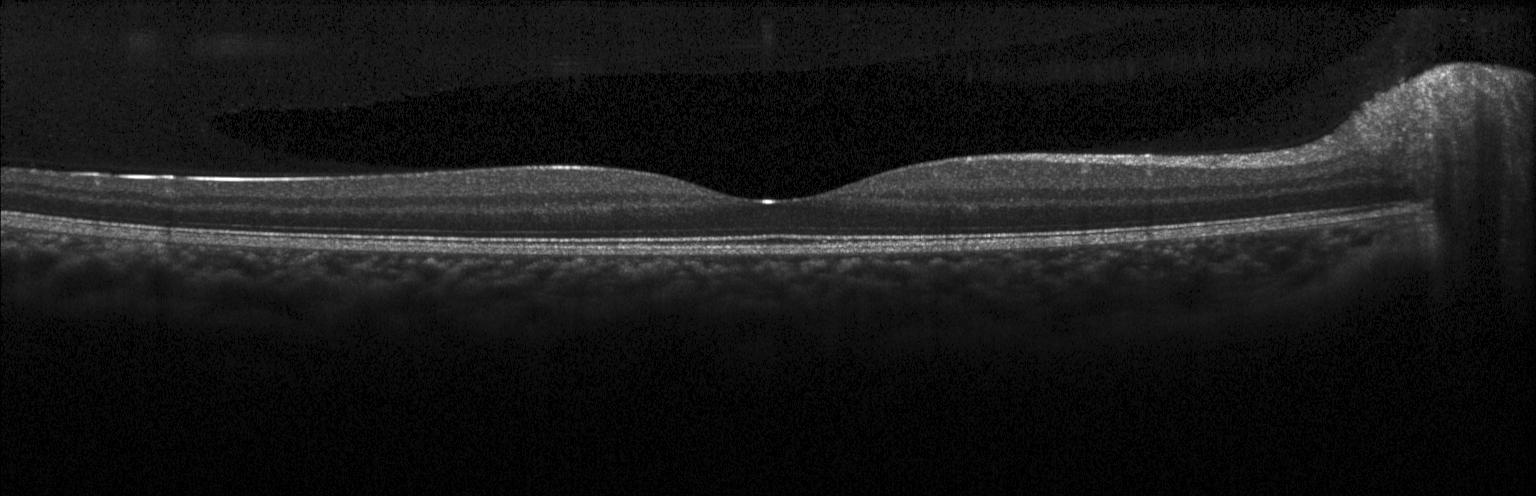 Impression: neither choroidal neovascularization, diabetic macular edema, nor drusen.